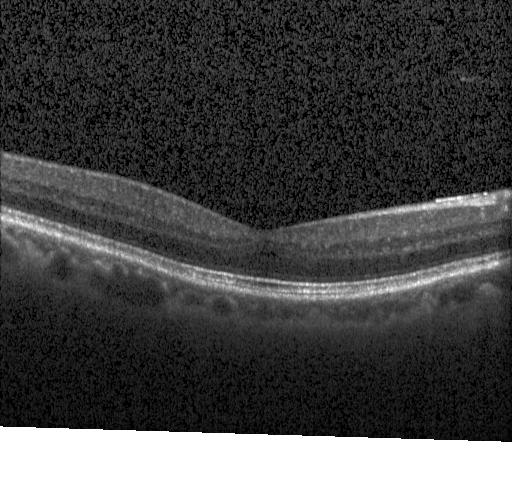

Assessment: neither choroidal neovascularization, diabetic macular edema, nor drusen.